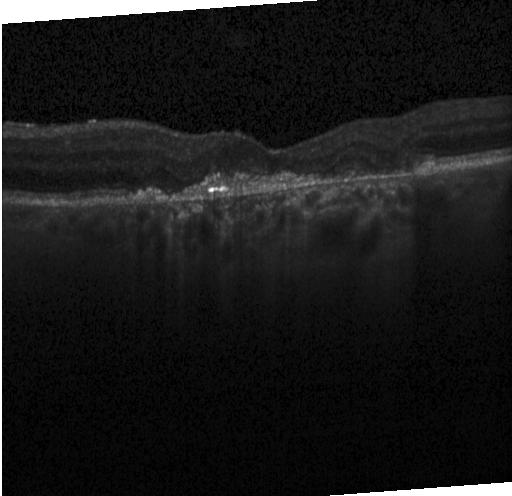 Retinal OCT B-scan.
Impression: a choroidal neovascular membrane.